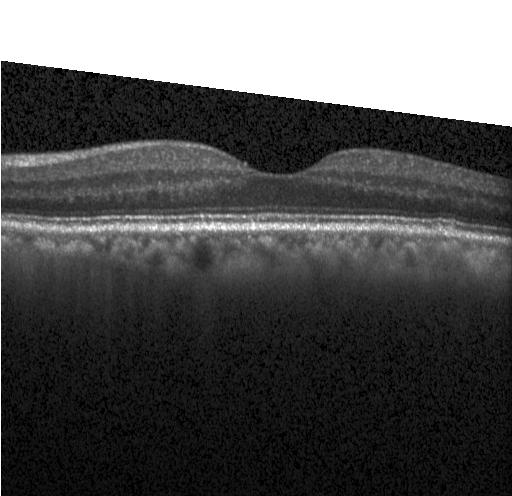 Fovea-centered. OCT B-scan
Diagnosis: no CNV, DME, or drusen.